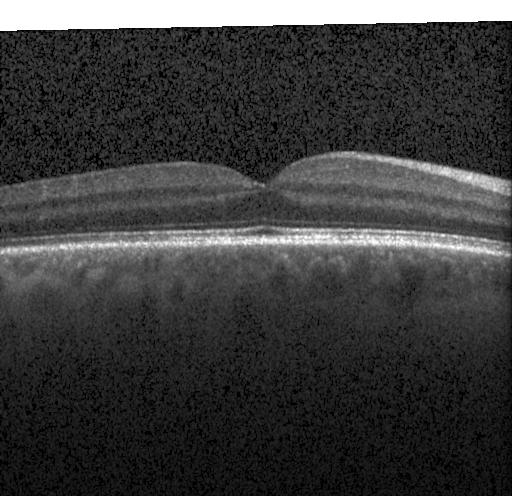
Acquired on a Heidelberg Spectralis · centered on the fovea · OCT line scan · spectral-domain optical coherence tomography — Macular OCT: no choroidal neovascularization, no diabetic macular edema, and no drusen.